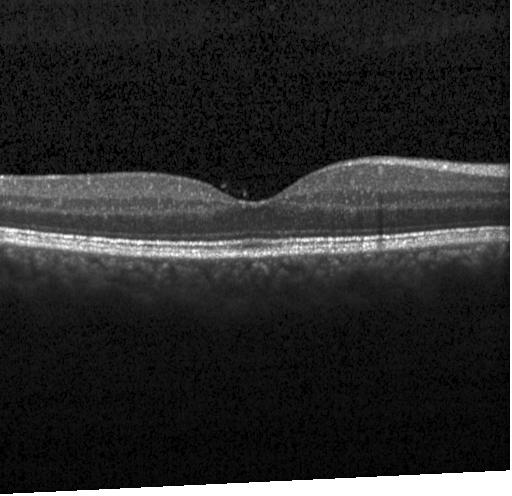

Spectral-domain OCT B-scan: no evidence of choroidal neovascularization, diabetic macular edema, or drusen.